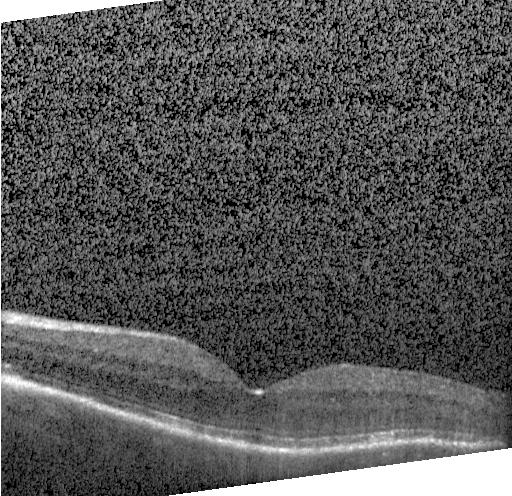 The scan shows no choroidal neovascularization, diabetic macular edema, or drusen.